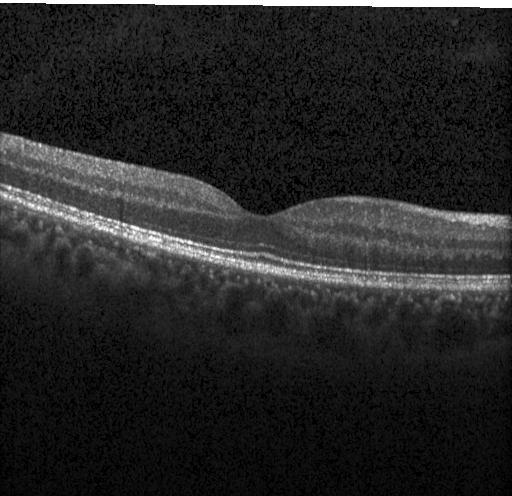 The scan shows neither CNV, DME, nor drusen.